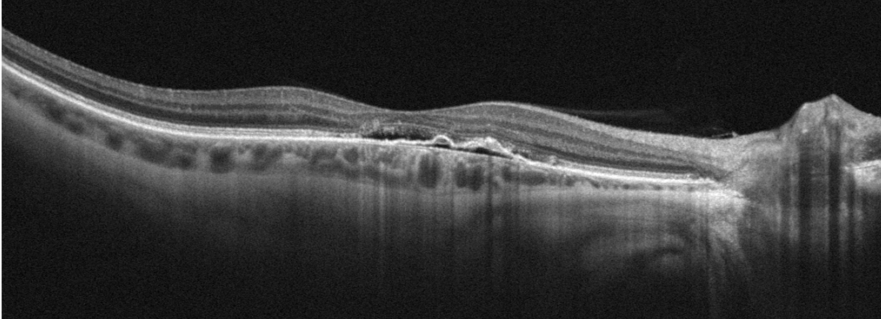

Acquired on an Optovue Avanti RTVue XR. Optical coherence tomography scan. Through the macula — Dx: AMD.